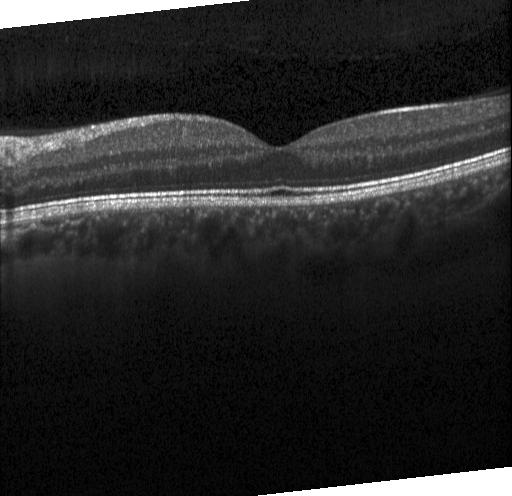 Finding: no choroidal neovascularization, diabetic macular edema, or drusen.